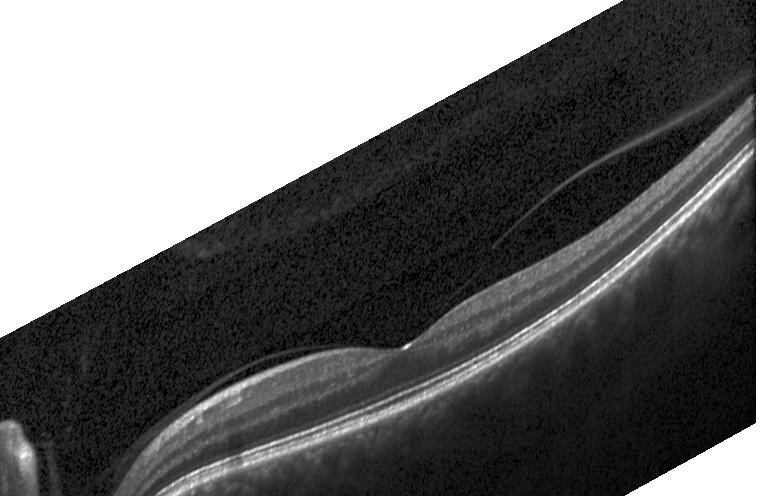

OCT line scan, Heidelberg Spectralis.
The scan shows no choroidal neovascularization, no diabetic macular edema, and no drusen.